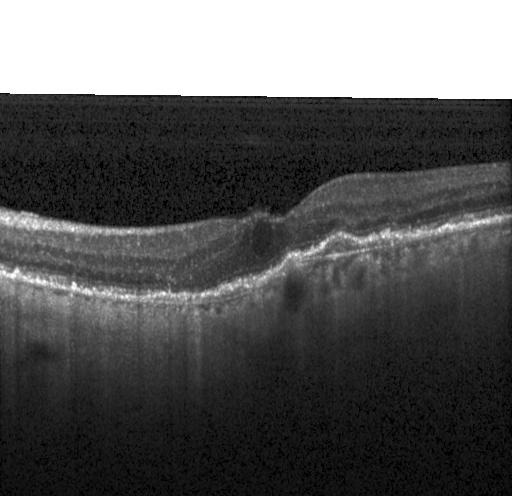

Retinal OCT cross-section
Finding: choroidal neovascularization (CNV).